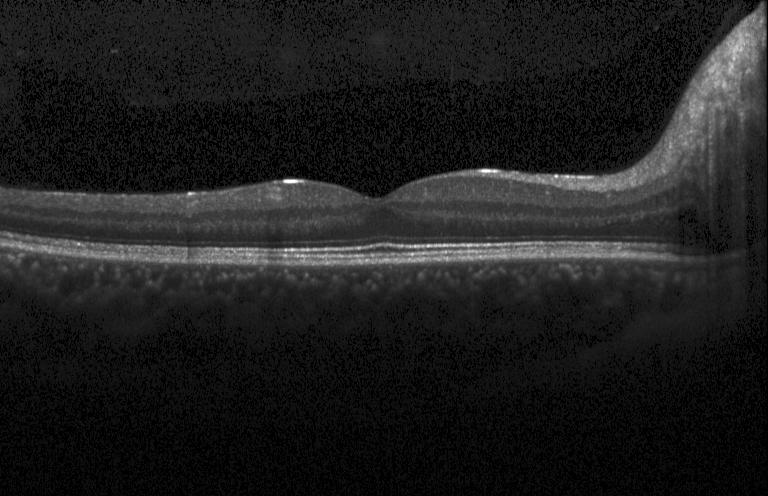
Optical coherence tomography B-scan, spectral-domain OCT. This B-scan demonstrates no choroidal neovascularization, no diabetic macular edema, and no drusen.